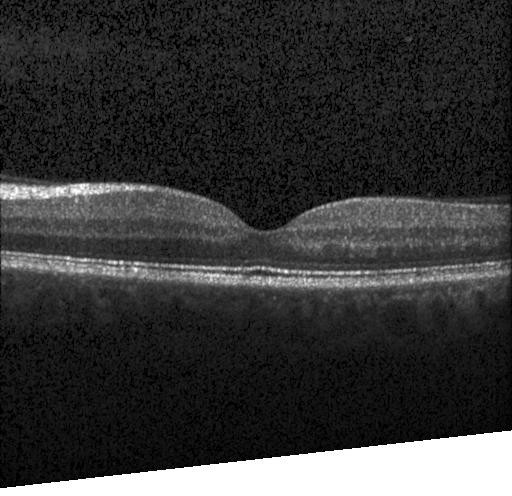

OCT line scan
Impression: no choroidal neovascularization, no diabetic macular edema, and no drusen.